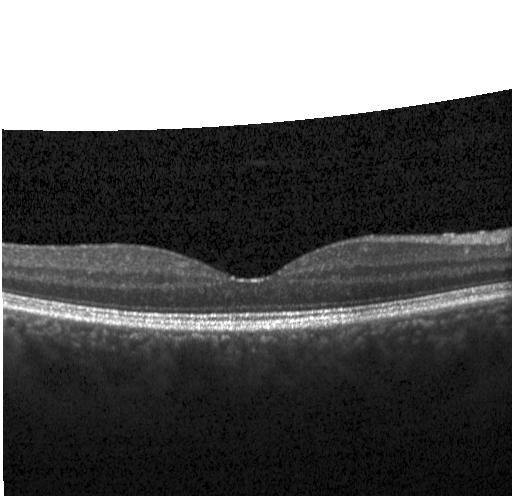

Spectral-domain optical coherence tomography, retinal OCT B-scan
Macular OCT: no evidence of CNV, DME, or drusen.